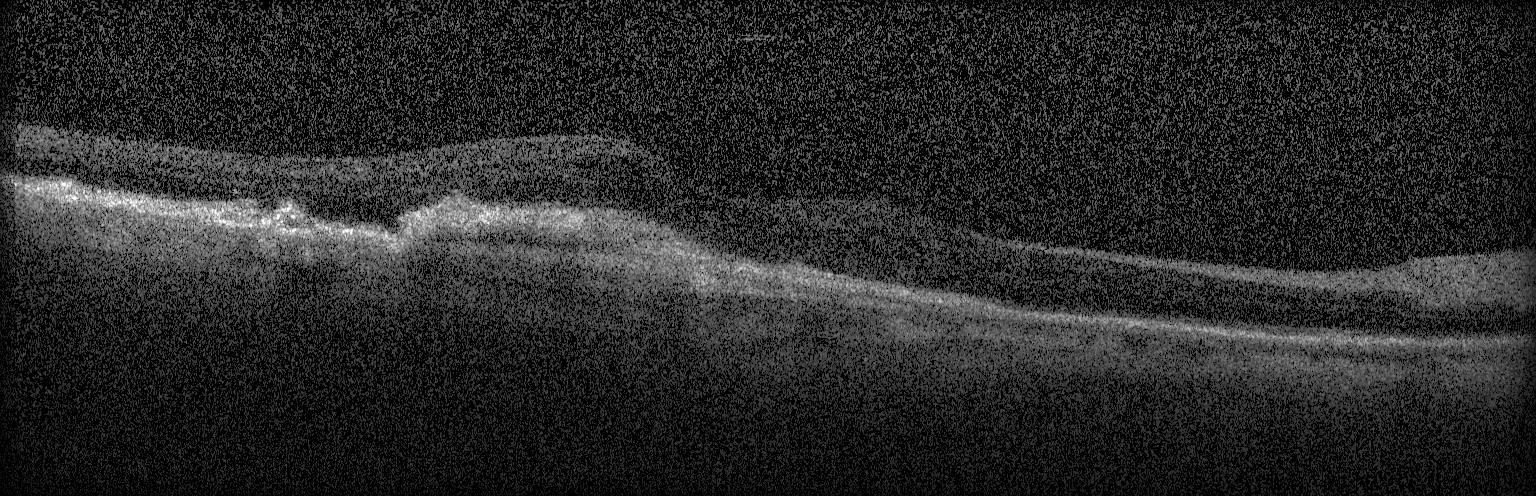
Optical coherence tomography scan; macular scan
Impression: a choroidal neovascular membrane.